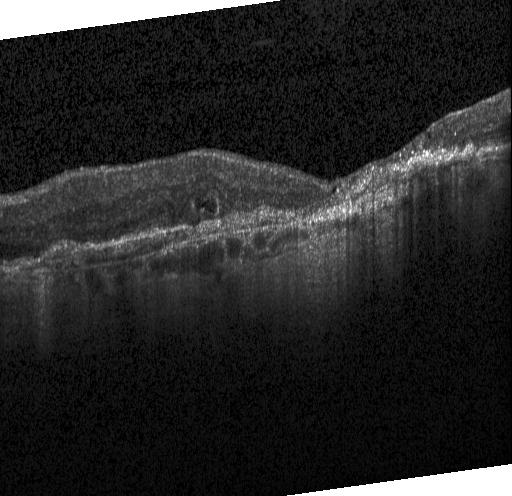
Choroidal neovascularization.